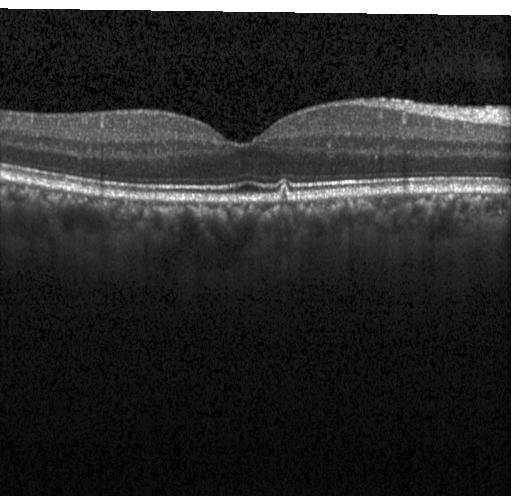 Optical coherence tomography scan
OCT finding: multiple drusen.